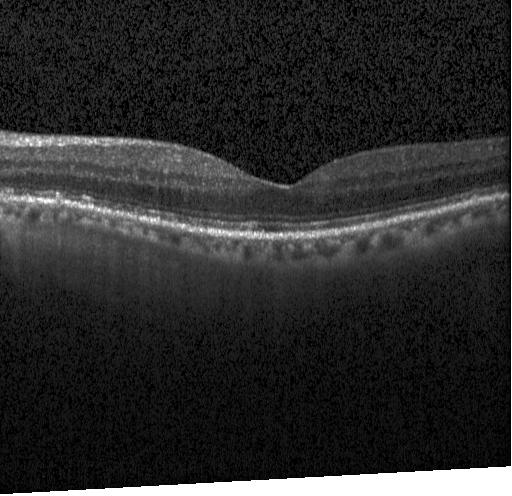 Impression: no evidence of choroidal neovascularization, diabetic macular edema, or drusen.